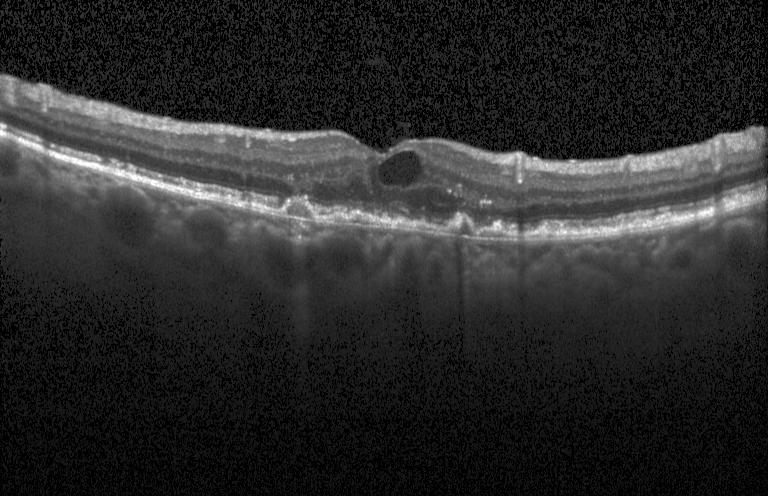
Diagnosis: a choroidal neovascular membrane.